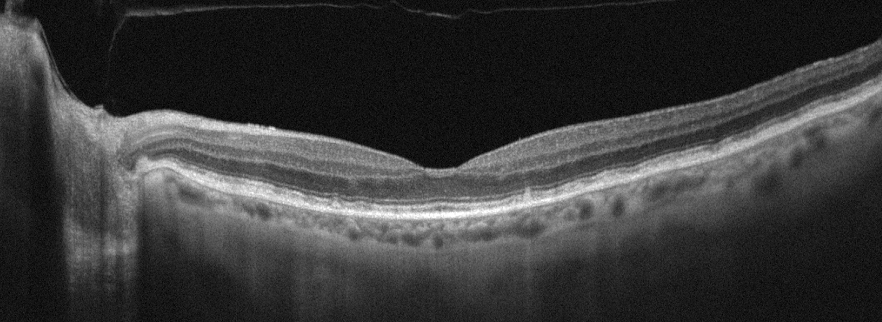 Instrument: Optovue Avanti RTVue XR. OCT B-scan.
Diagnosis: age-related macular degeneration (AMD).